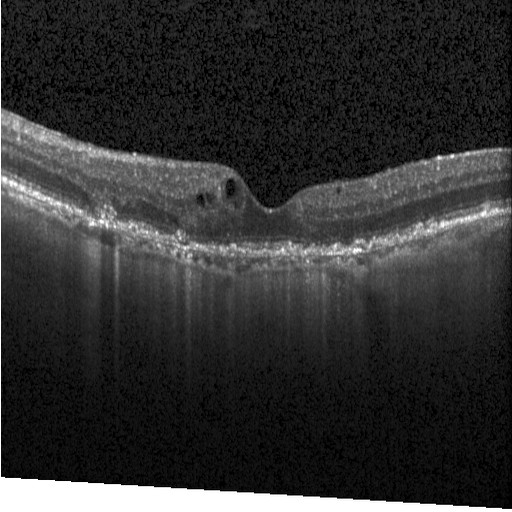

Spectral-domain optical coherence tomography; optical coherence tomography scan
Macular OCT: diabetic macular edema (DME).